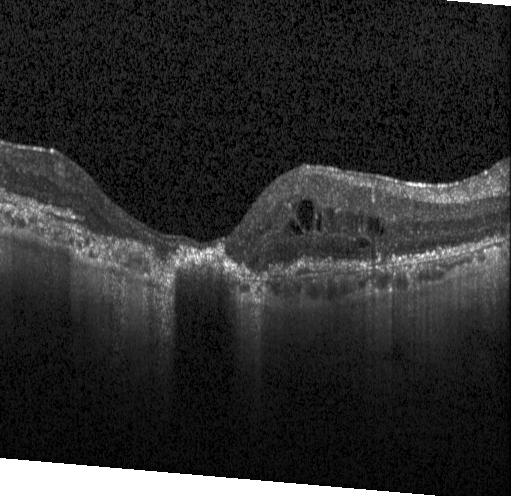 Retinal OCT B-scan. Assessment: a choroidal neovascular membrane.